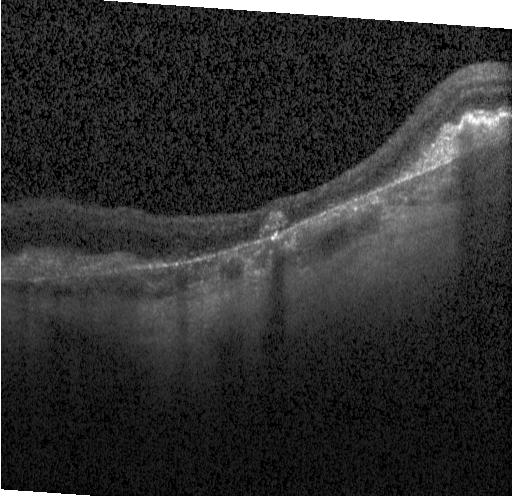

OCT B-scan
Assessment: choroidal neovascularization.